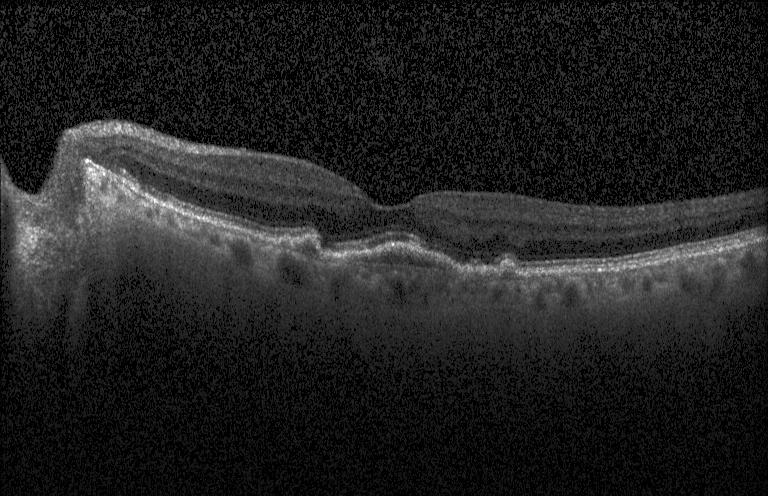

Acquired on a Heidelberg Spectralis, retinal OCT B-scan
OCT finding: choroidal neovascularization.